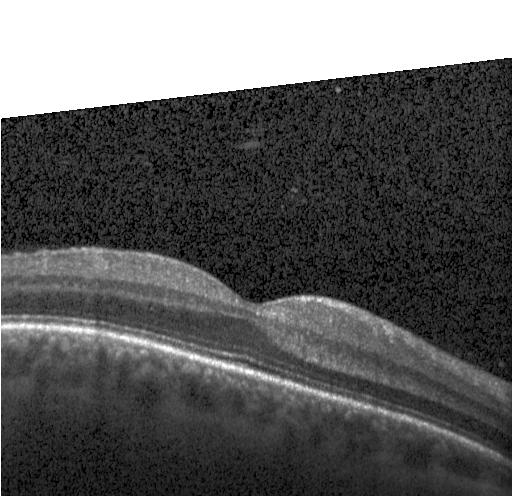

OCT B-scan; acquired on a Heidelberg Spectralis; fovea-centered
Finding: neither CNV, DME, nor drusen.